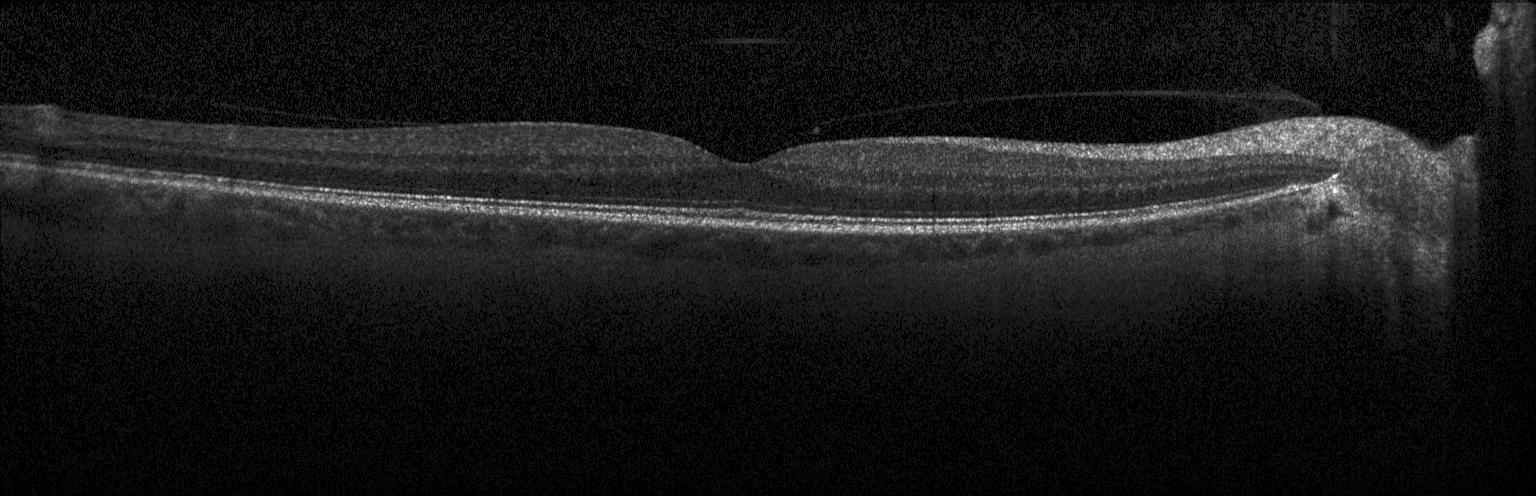 Optical coherence tomography B-scan; spectral-domain OCT.
Diagnosis: no evidence of choroidal neovascularization, diabetic macular edema, or drusen.